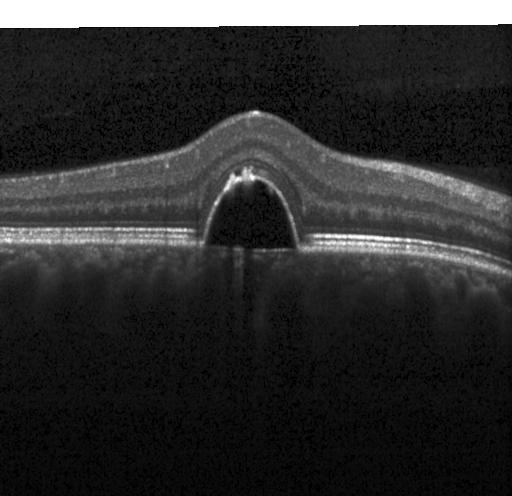 Instrument: Heidelberg Spectralis; retinal OCT cross-section; spectral-domain OCT; centered on the fovea.
The scan shows choroidal neovascularization (CNV).